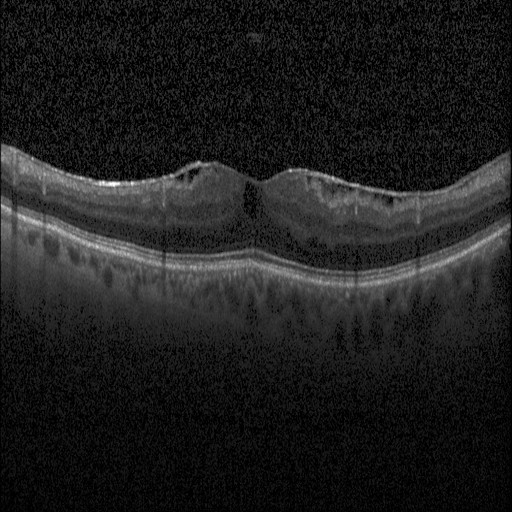 Fovea-centered · Heidelberg Spectralis · optical coherence tomography B-scan
The scan shows diabetic macular edema.